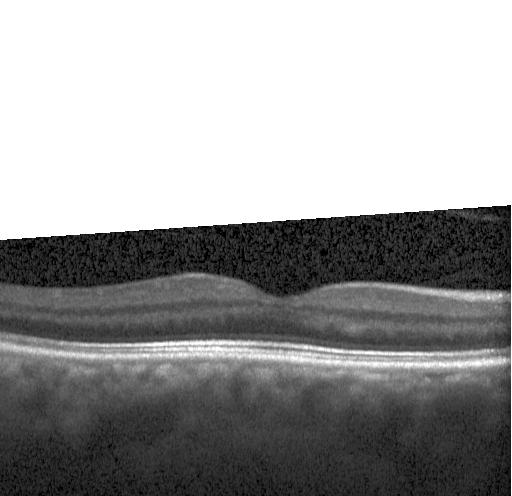
Optical coherence tomography B-scan. Diagnosis: no evidence of CNV, DME, or drusen.